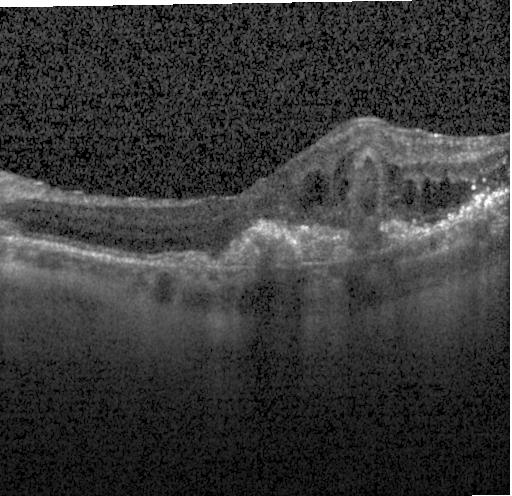
Spectral-domain OCT, acquired on a Heidelberg Spectralis, retinal OCT cross-section — Impression: CNV.